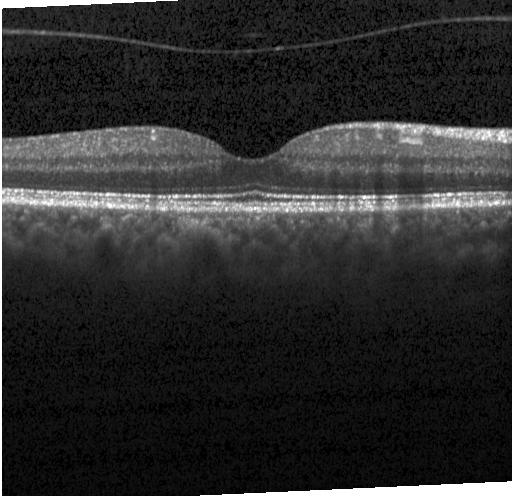

Dx: no choroidal neovascularization, diabetic macular edema, or drusen.